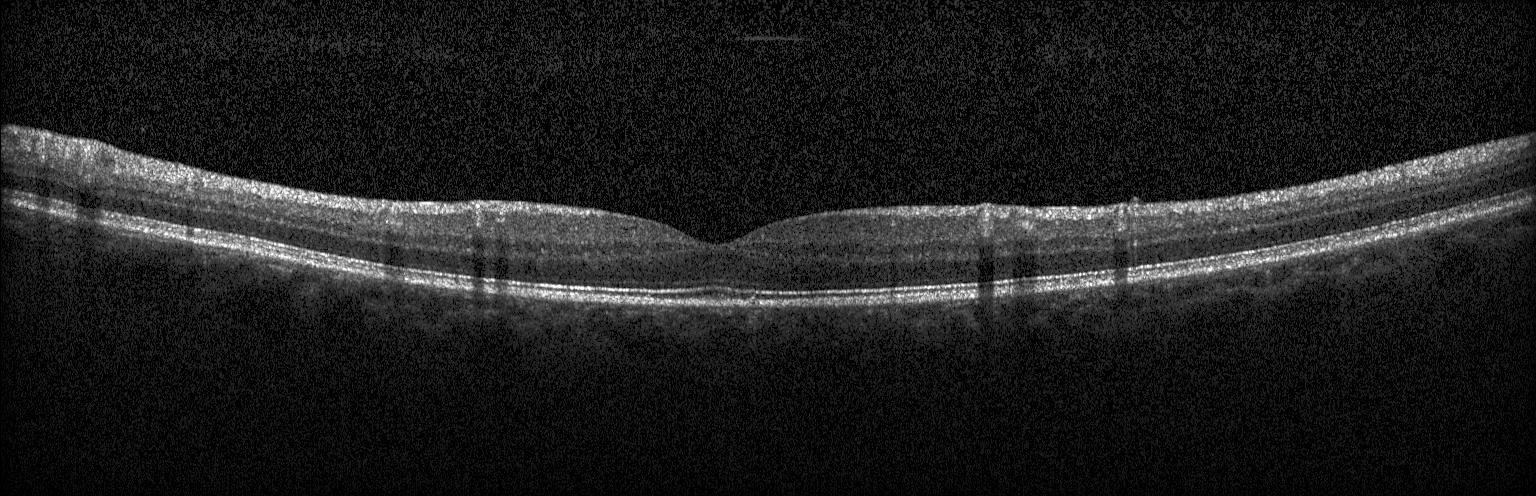 Optical coherence tomography scan
Diagnosis: neither choroidal neovascularization, diabetic macular edema, nor drusen.